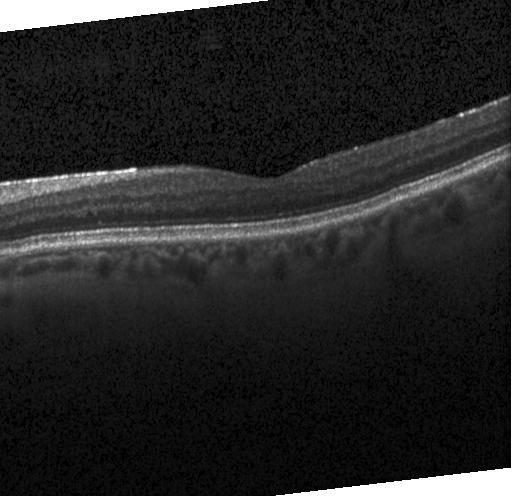 Spectral-domain OCT; Heidelberg Spectralis OCT system; optical coherence tomography B-scan; macular scan.
The scan shows neither CNV, DME, nor drusen.